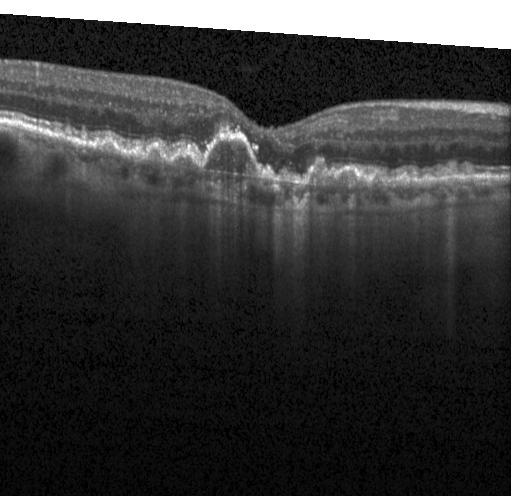
Retinal OCT B-scan. Impression: a choroidal neovascular membrane.